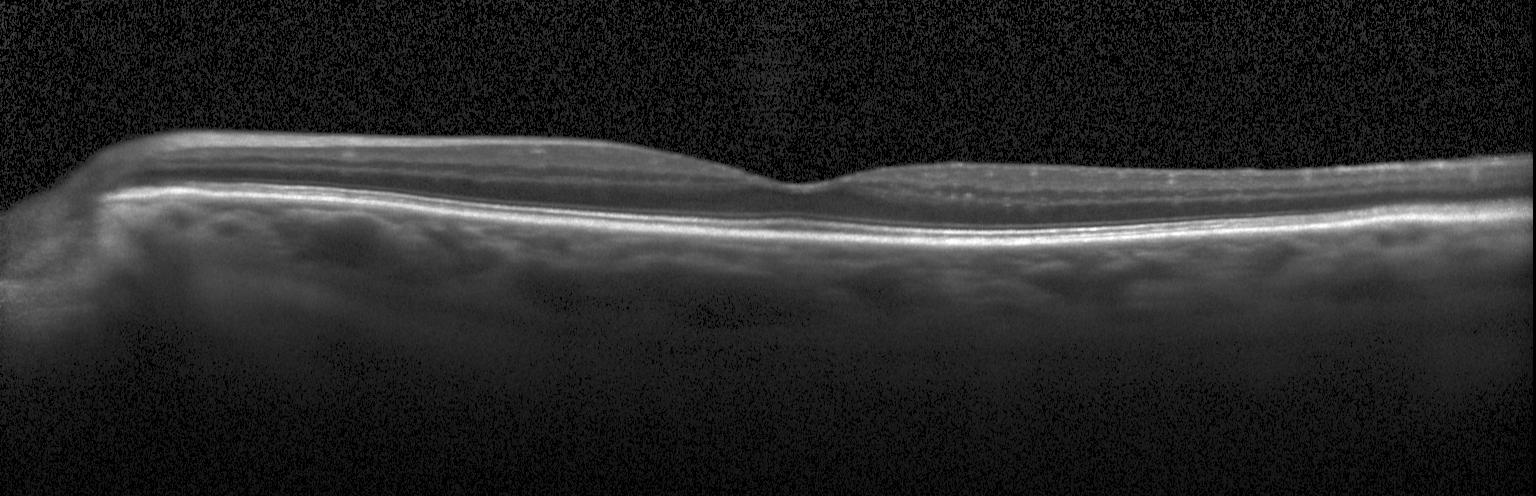
Retinal OCT B-scan. The scan shows no CNV, no DME, and no drusen.